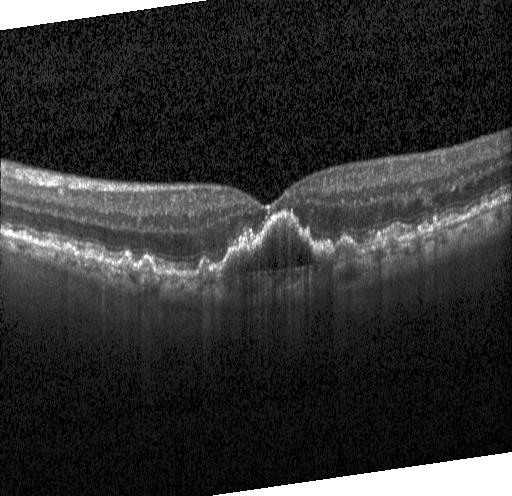

CNV.